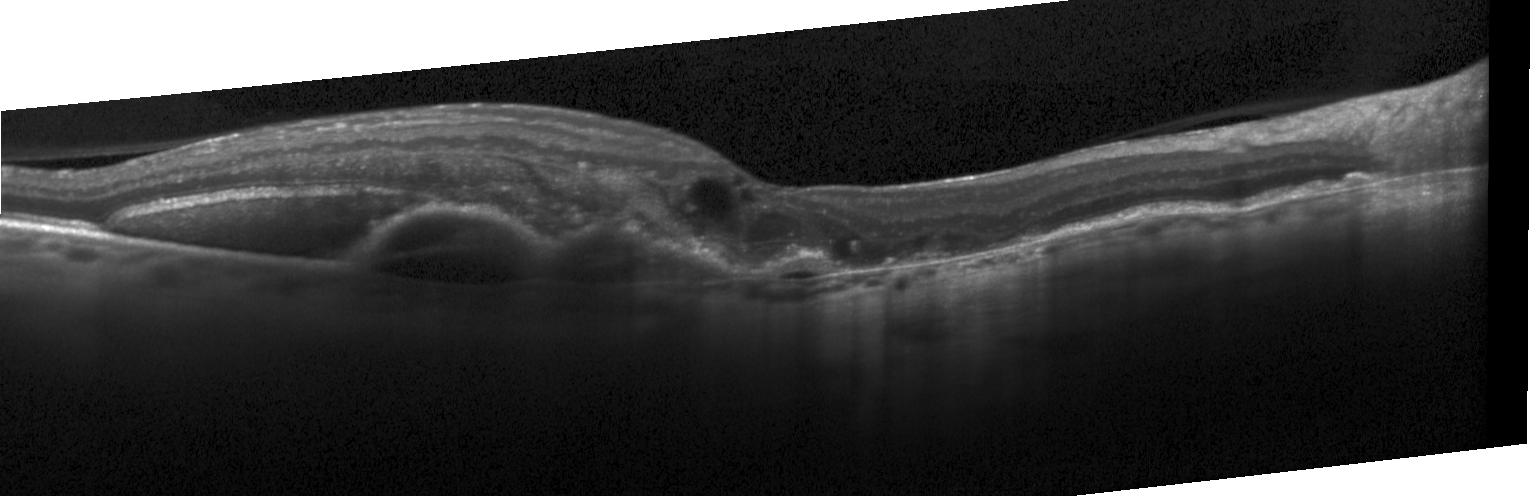

Assessment: choroidal neovascularization (CNV).